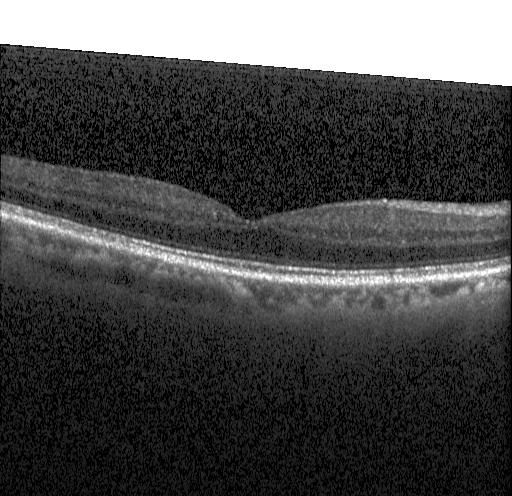 Macular scan. Spectral-domain OCT. OCT line scan — Impression: no evidence of CNV, DME, or drusen.